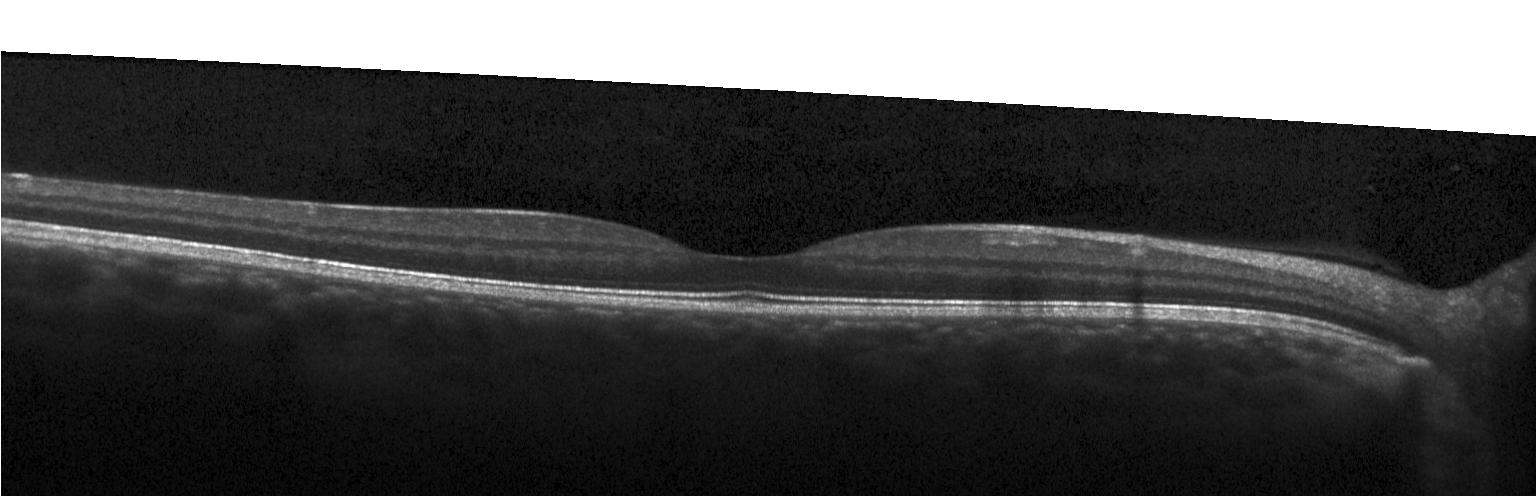

OCT B-scan. Assessment: no choroidal neovascularization, diabetic macular edema, or drusen.